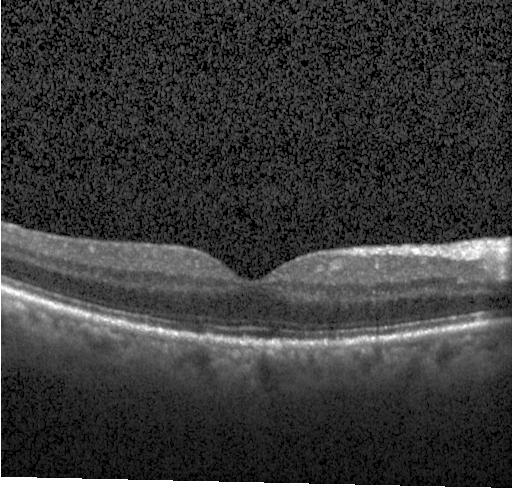 Impression: no evidence of choroidal neovascularization, diabetic macular edema, or drusen.